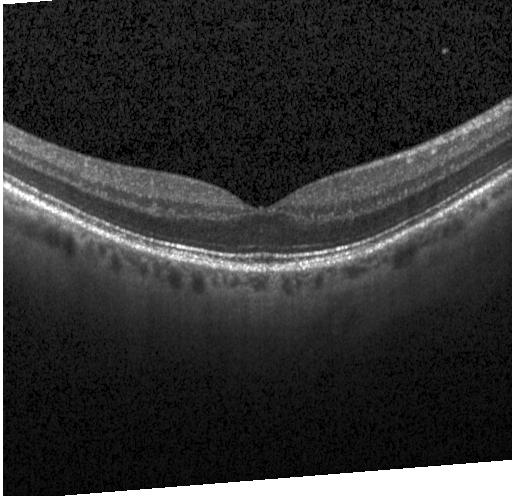
Heidelberg Spectralis OCT system, retinal OCT B-scan, centered on the fovea, spectral-domain OCT — Impression: no CNV, no DME, and no drusen.